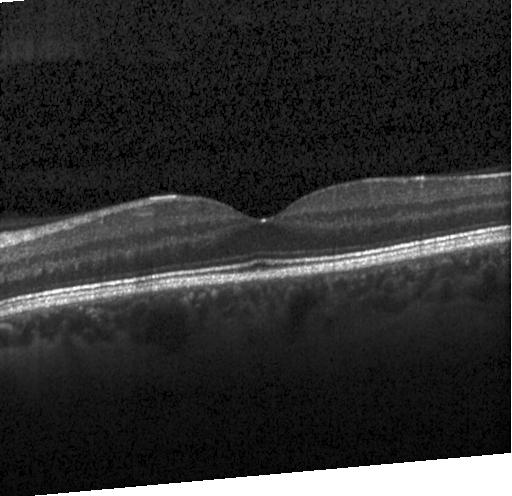

Spectral-domain optical coherence tomography; OCT line scan; acquired on a Heidelberg Spectralis; fovea-centered — Finding: neither choroidal neovascularization, diabetic macular edema, nor drusen.